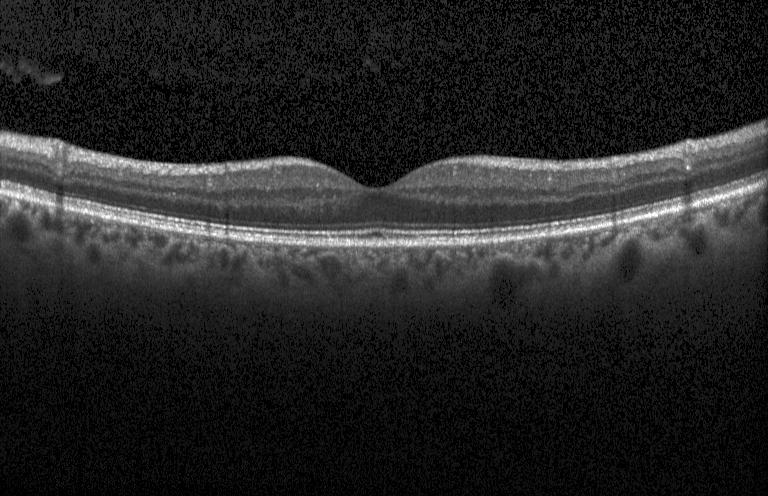 Optical coherence tomography B-scan; acquired on a Heidelberg Spectralis — Assessment: neither choroidal neovascularization, diabetic macular edema, nor drusen.